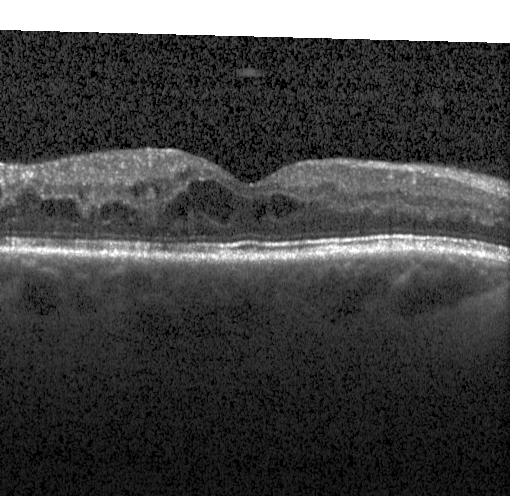

Optical coherence tomography B-scan, spectral-domain OCT. Impression: diabetic macular edema.